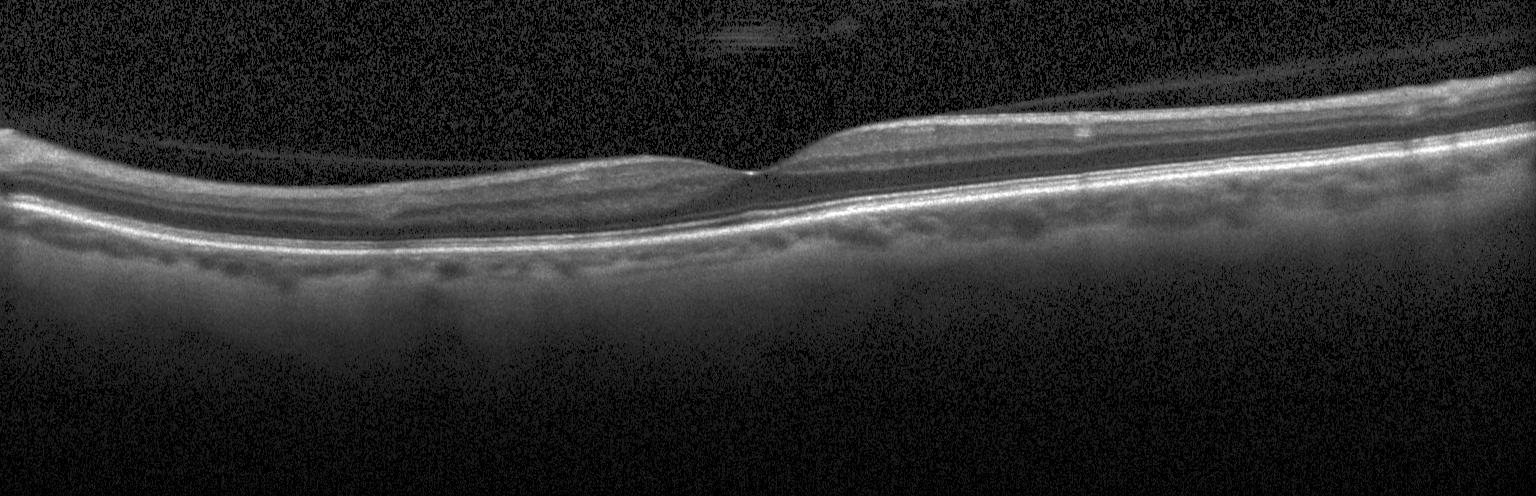

Dx: no choroidal neovascularization, diabetic macular edema, or drusen.